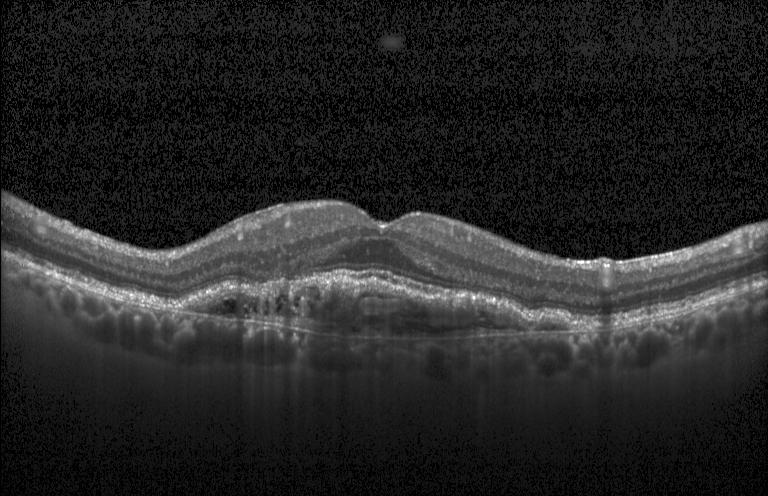

Dx: a choroidal neovascular membrane.